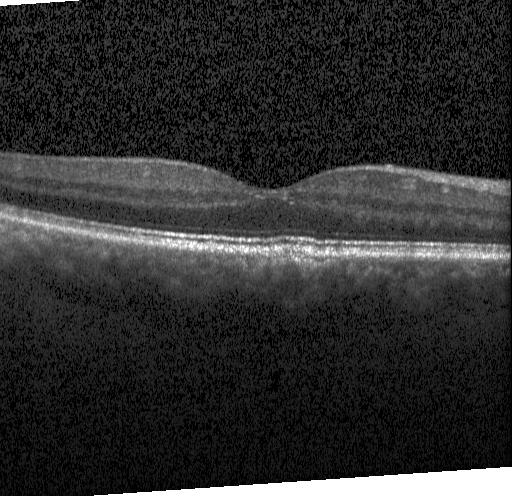 Centered on the fovea · SD-OCT · retinal OCT cross-section
Assessment: no choroidal neovascularization, diabetic macular edema, or drusen.